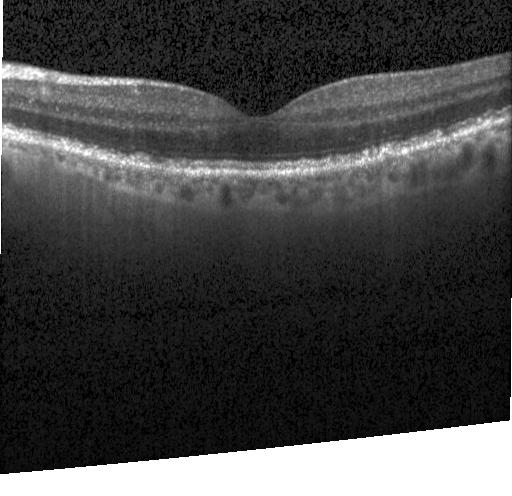 OCT line scan. Instrument: Heidelberg Spectralis
Sub-RPE drusenoid deposits.